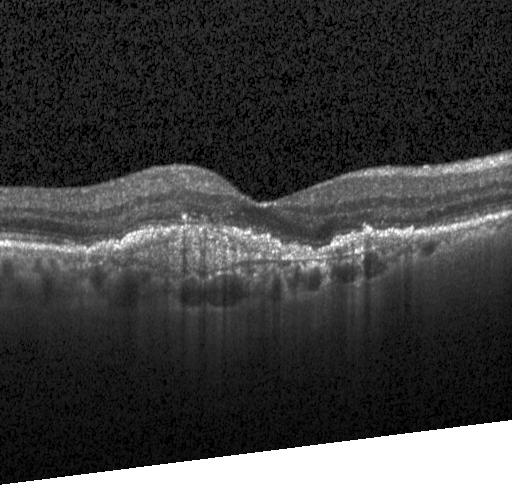

OCT B-scan showing a choroidal neovascular membrane.